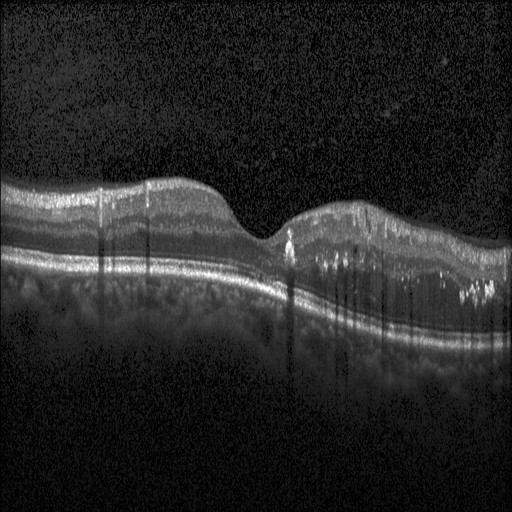 The scan shows diabetic macular edema (DME).